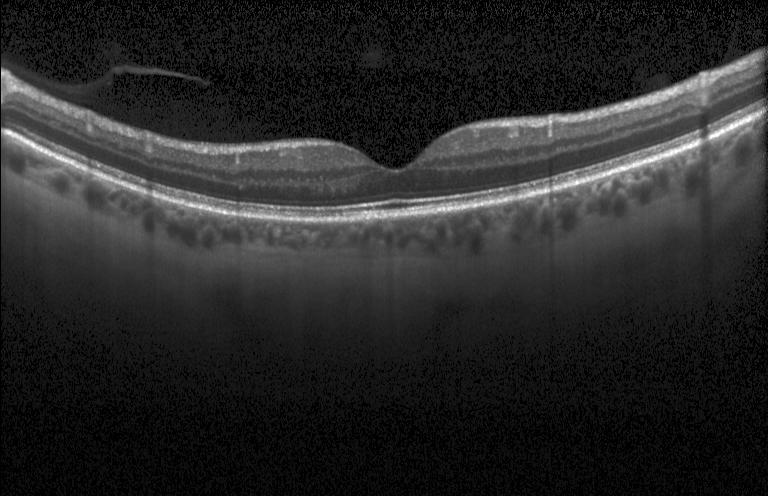

Heidelberg Spectralis OCT system; spectral-domain optical coherence tomography; retinal OCT B-scan; horizontal scan through the fovea
This B-scan demonstrates neither choroidal neovascularization, diabetic macular edema, nor drusen.